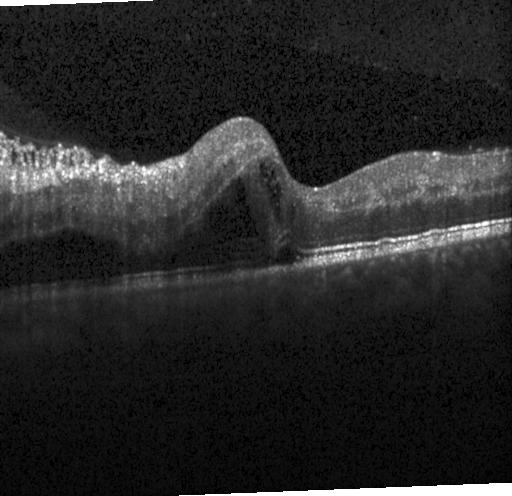

OCT line scan
Dx: diabetic macular edema.